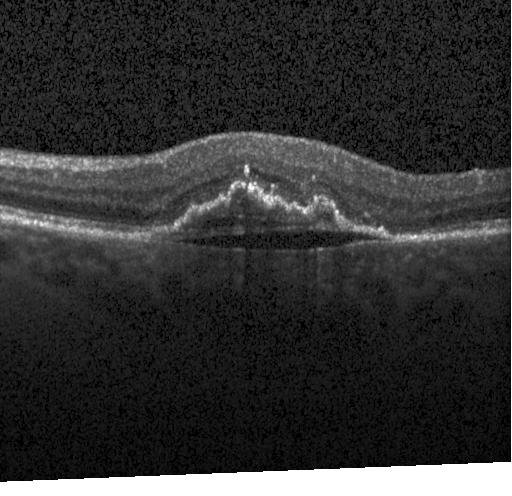
Assessment: choroidal neovascularization (CNV).